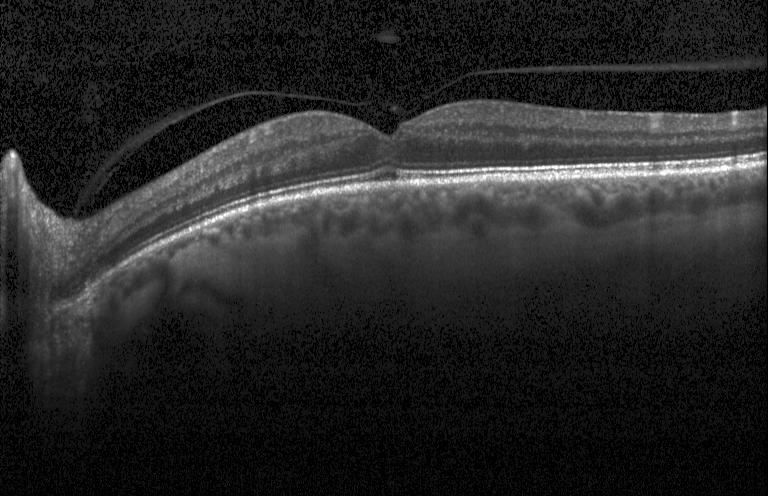
Retinal OCT cross-section showing neither choroidal neovascularization, diabetic macular edema, nor drusen.